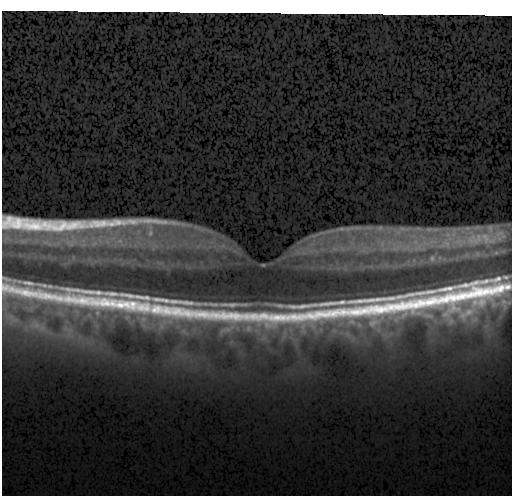 Spectral-domain OCT; optical coherence tomography B-scan; acquired on a Heidelberg Spectralis
Assessment: no evidence of CNV, DME, or drusen.